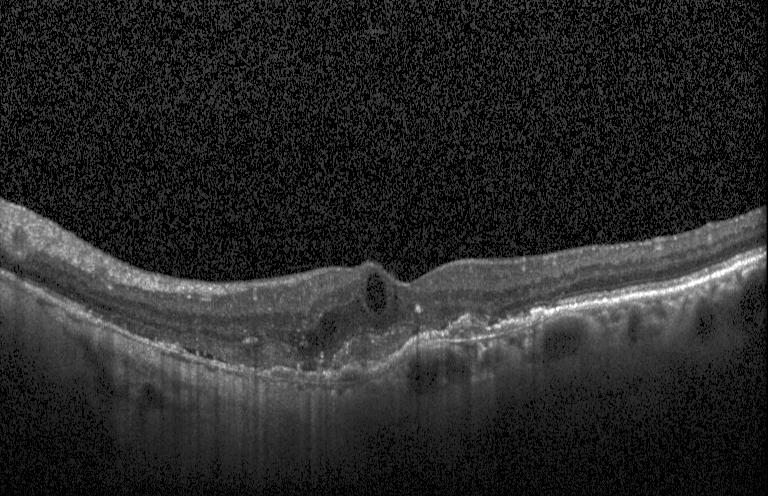 This B-scan demonstrates a choroidal neovascular membrane.